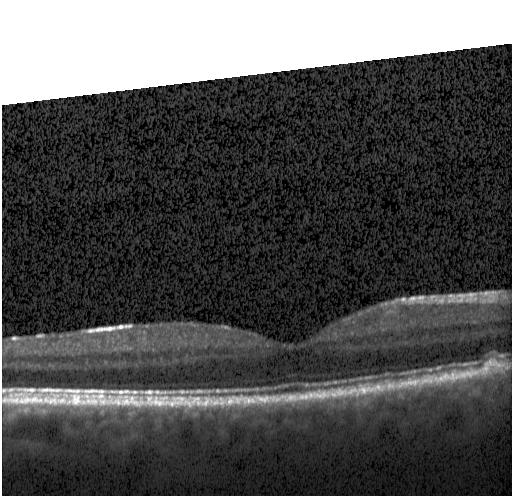 Retinal OCT B-scan.
Macular OCT: multiple drusen.